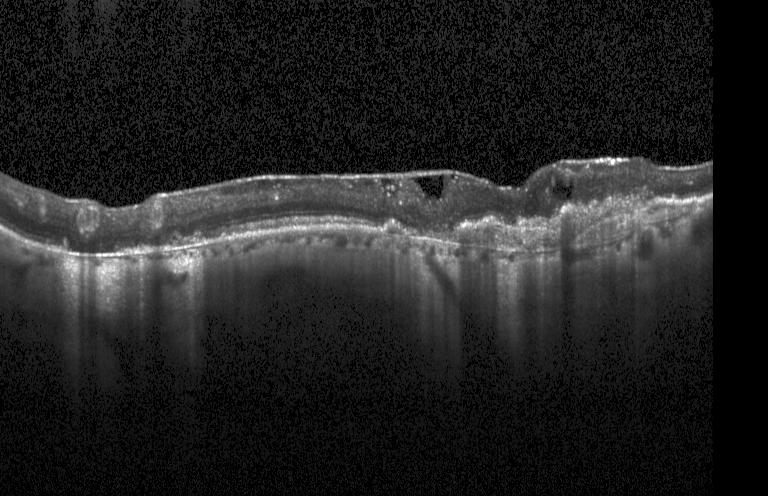 Retinal OCT cross-section; spectral-domain optical coherence tomography; through the macula.
Assessment: a choroidal neovascular membrane.